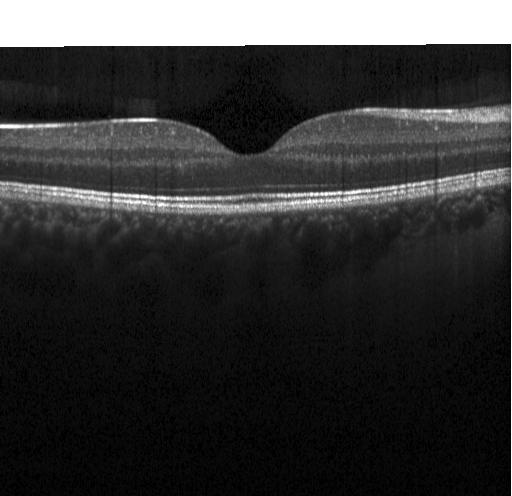 Impression: no choroidal neovascularization, no diabetic macular edema, and no drusen.